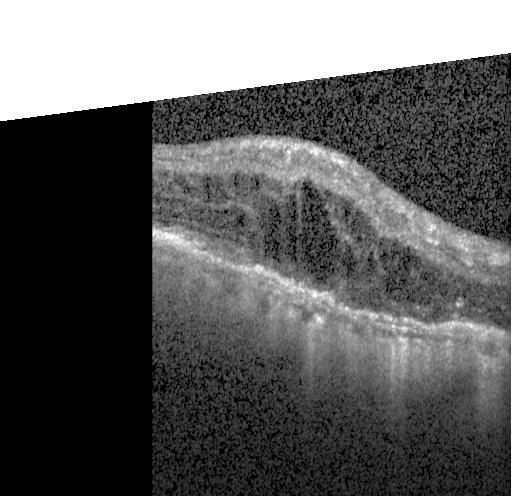
Spectral-domain optical coherence tomography; through the macula; Heidelberg Spectralis; optical coherence tomography B-scan
Assessment: a choroidal neovascular membrane.